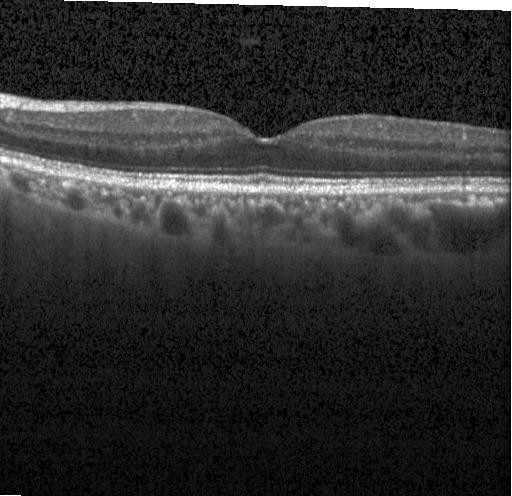

Horizontal scan through the fovea; OCT line scan — Impression: neither CNV, DME, nor drusen.